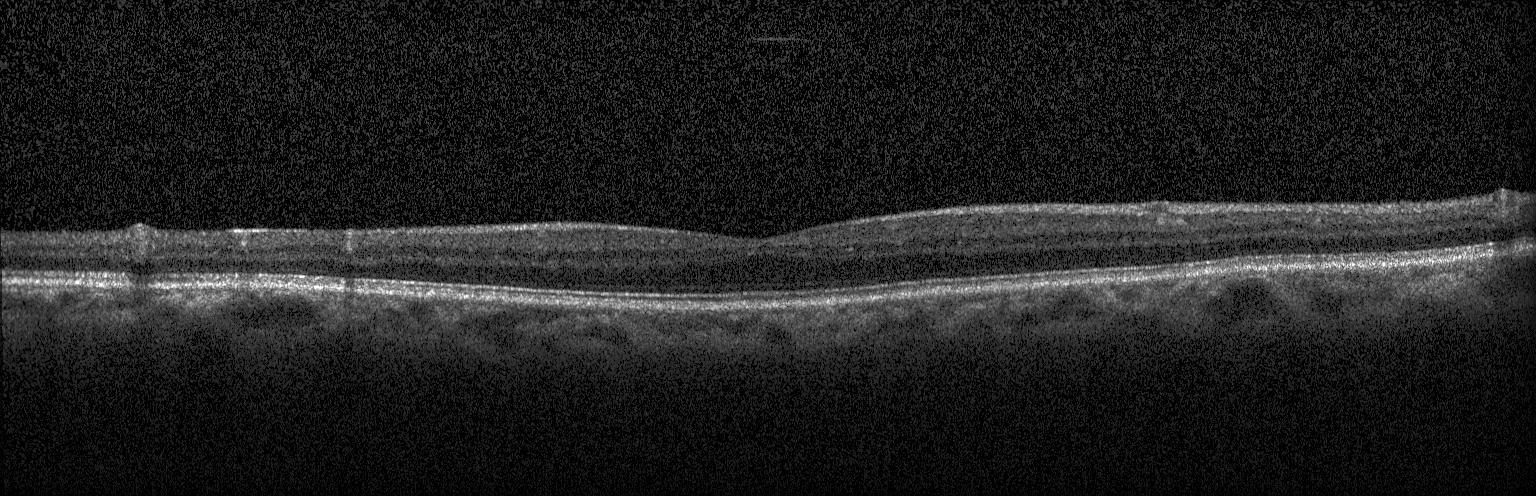 OCT B-scan showing no choroidal neovascularization, diabetic macular edema, or drusen.